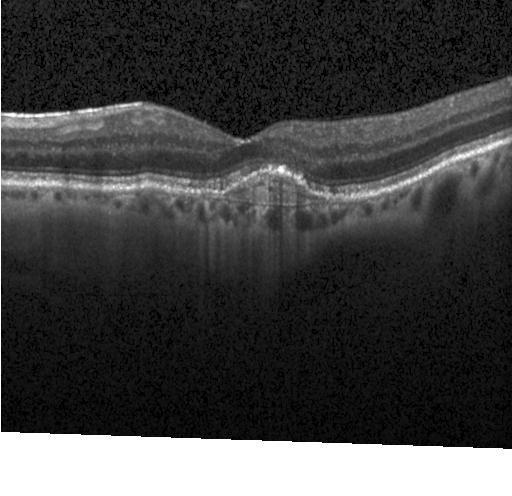 SD-OCT; OCT B-scan; macular scan
Macular OCT: a choroidal neovascular membrane.